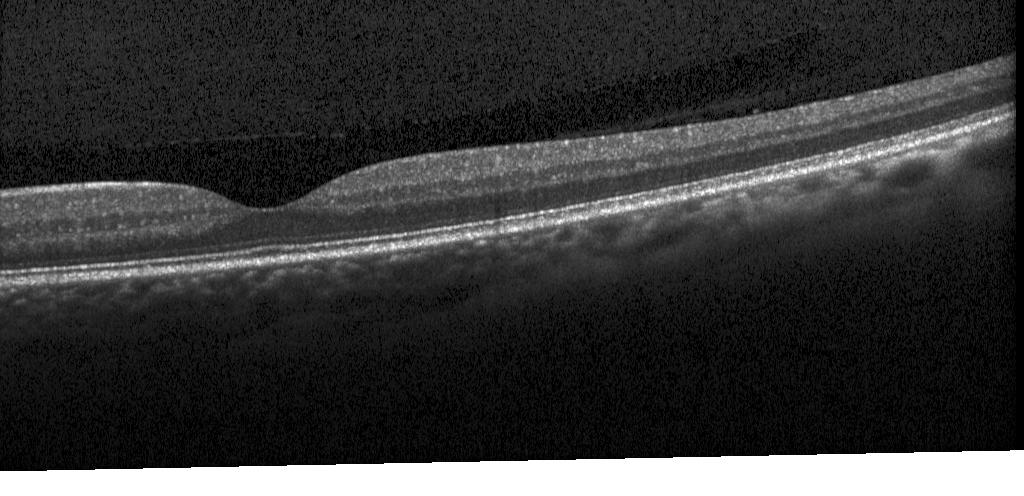
OCT B-scan — Dx: no evidence of CNV, DME, or drusen.